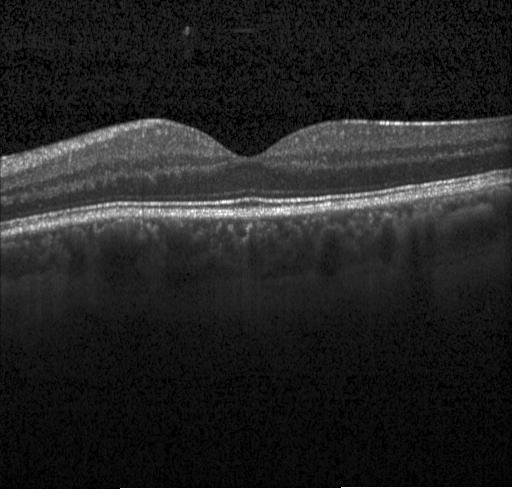
Fovea-centered. Retinal OCT B-scan. Instrument: Heidelberg Spectralis — Macular OCT: no CNV, no DME, and no drusen.